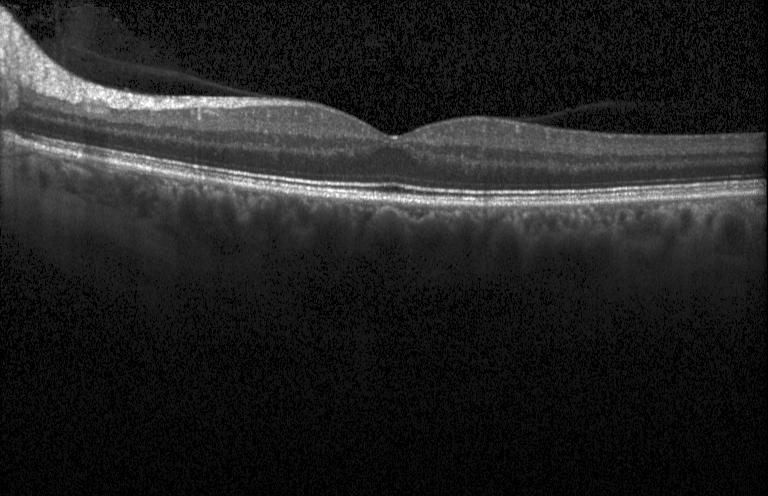

Impression: no choroidal neovascularization, diabetic macular edema, or drusen.